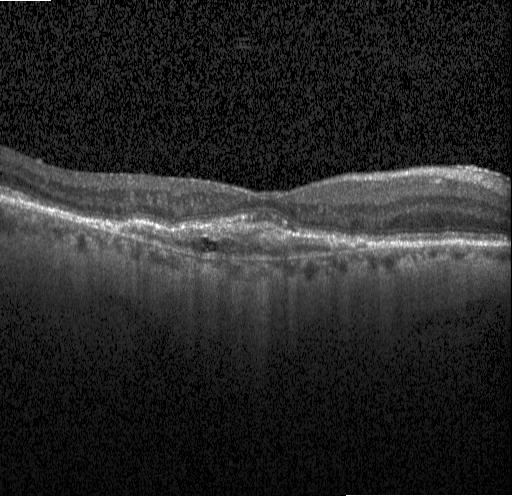
Optical coherence tomography B-scan; spectral-domain OCT; instrument: Heidelberg Spectralis — Impression: a choroidal neovascular membrane.